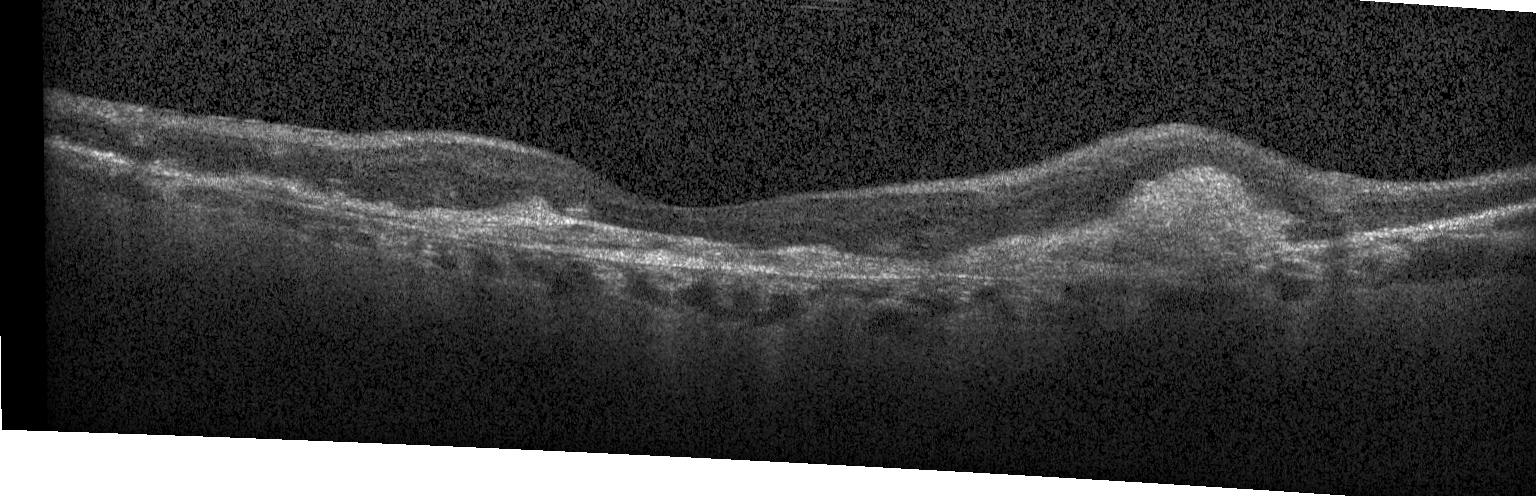 Retinal OCT cross-section; Heidelberg Spectralis; SD-OCT — OCT finding: choroidal neovascularization (CNV).